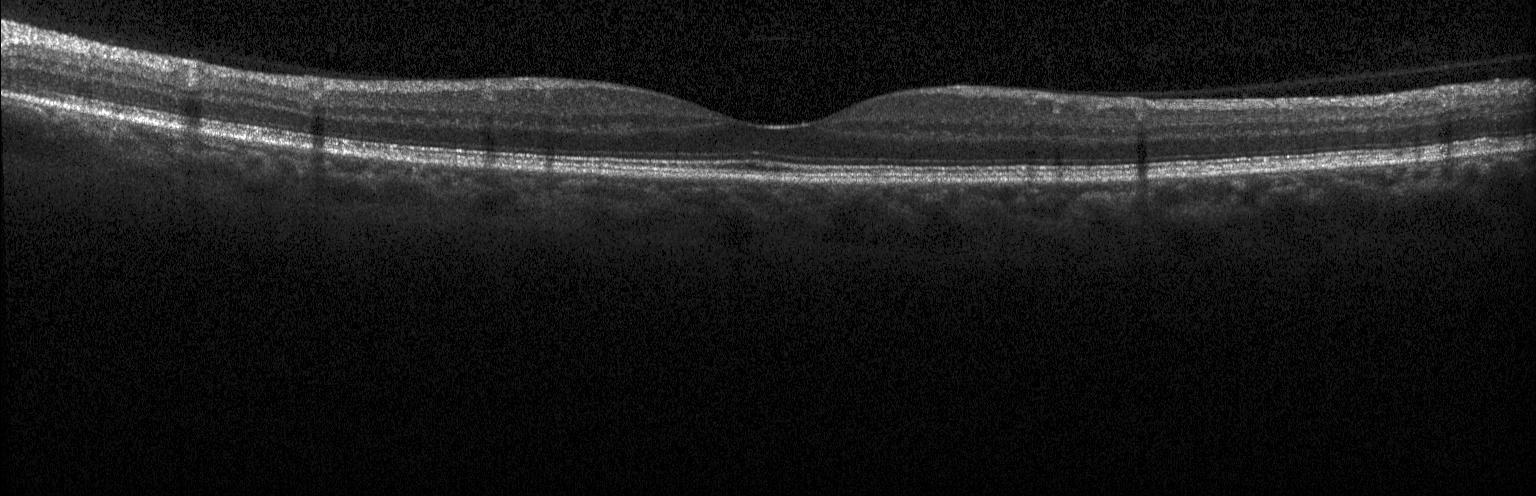 Retinal OCT cross-section showing no evidence of choroidal neovascularization, diabetic macular edema, or drusen.